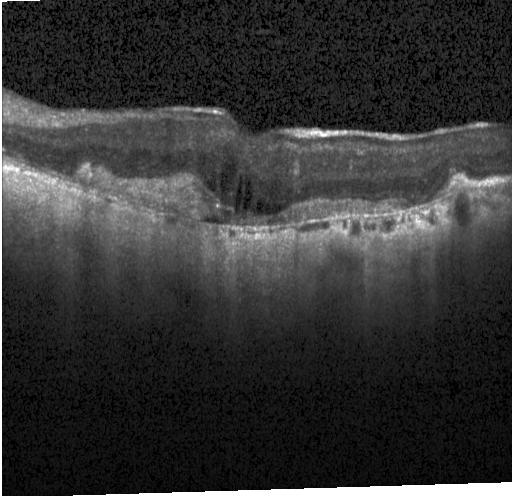
Optical coherence tomography scan. Spectral-domain OCT. Heidelberg Spectralis OCT system. Macular scan — Impression: choroidal neovascularization.